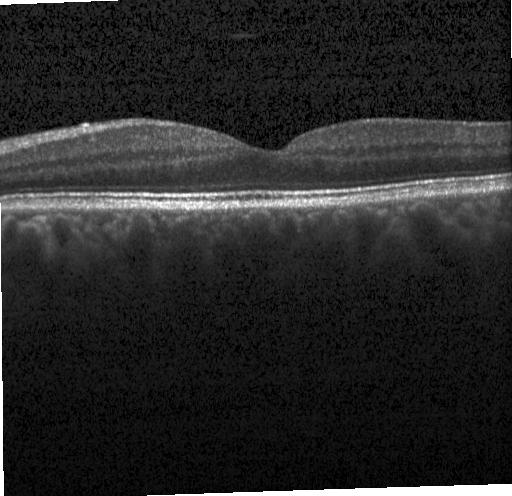 Dx: no CNV, no DME, and no drusen.